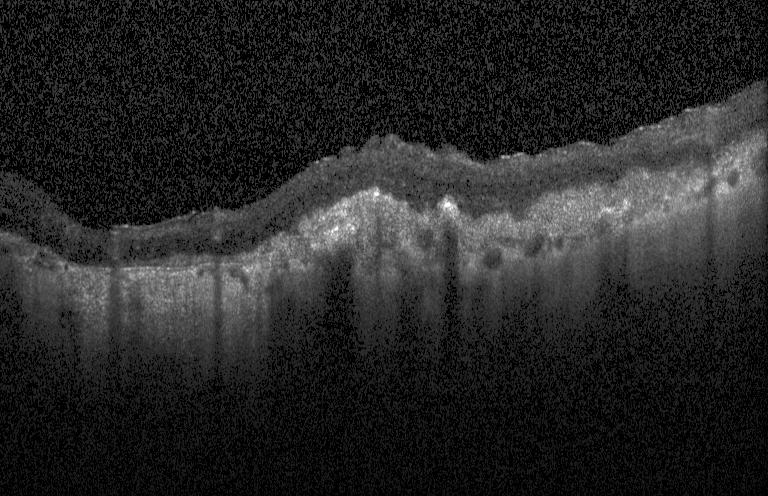 Spectral-domain optical coherence tomography, optical coherence tomography B-scan, horizontal scan through the fovea — Impression: a choroidal neovascular membrane.